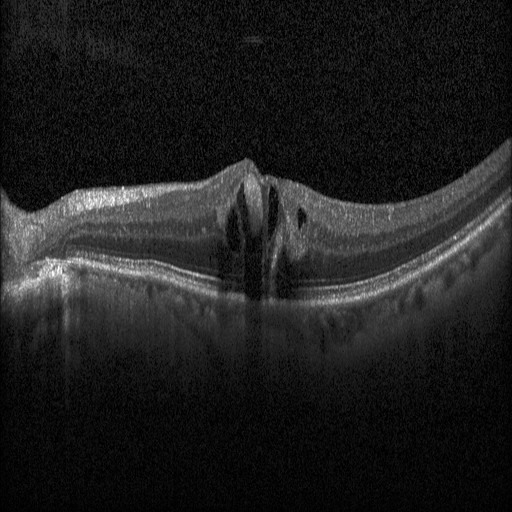
Diagnosis: diabetic macular edema.